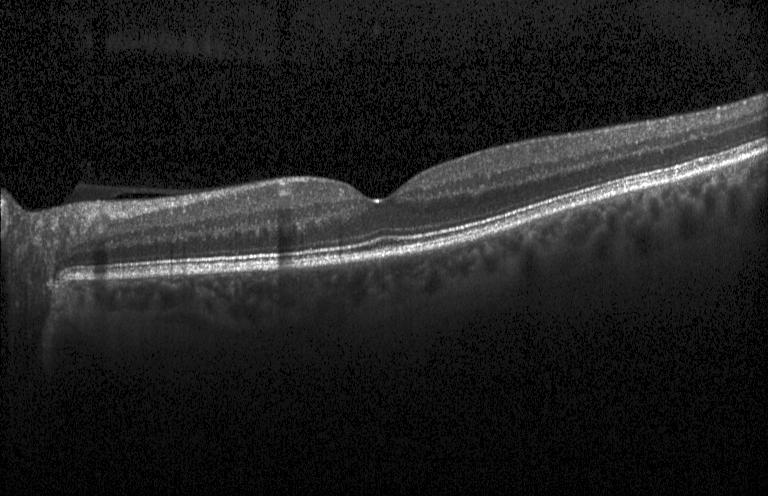 OCT B-scan
No choroidal neovascularization, no diabetic macular edema, and no drusen.